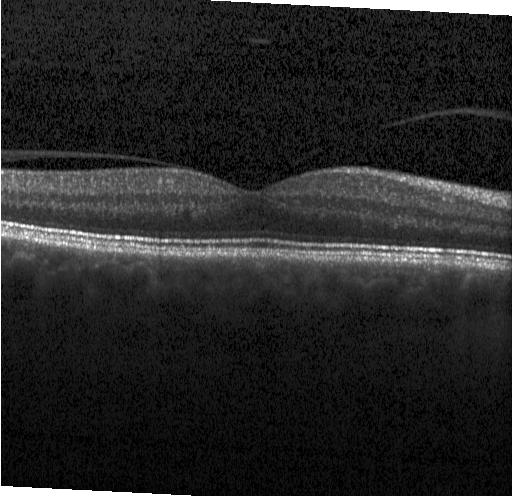
Optical coherence tomography B-scan.
Diagnosis: no CNV, no DME, and no drusen.